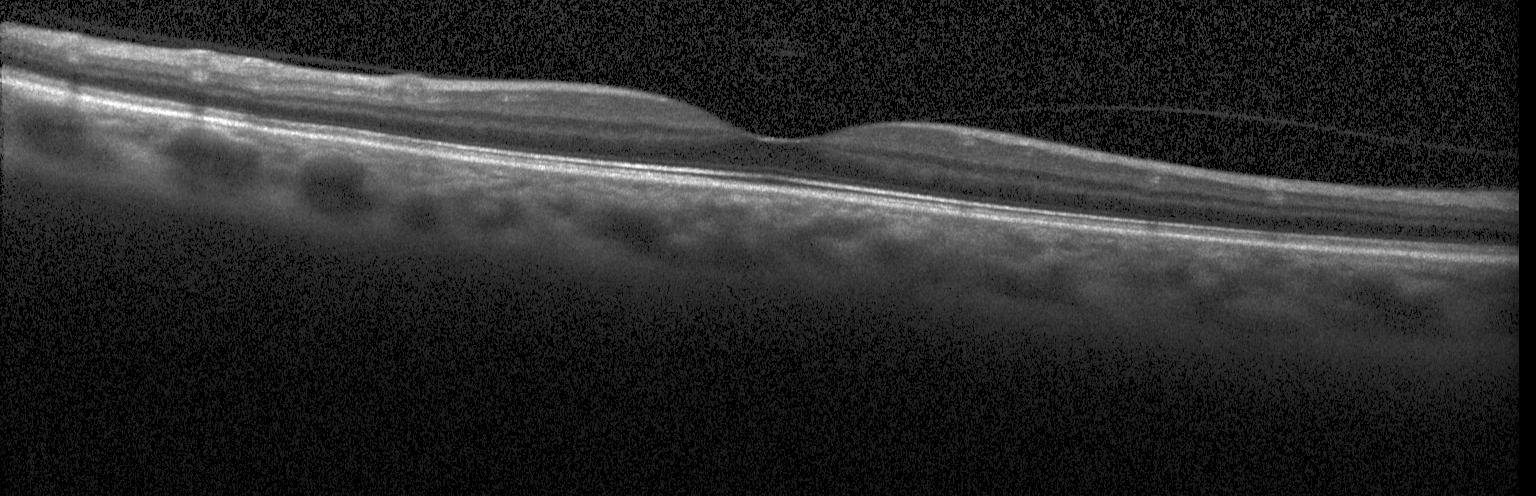
Macular scan; SD-OCT; optical coherence tomography scan.
The scan shows neither choroidal neovascularization, diabetic macular edema, nor drusen.